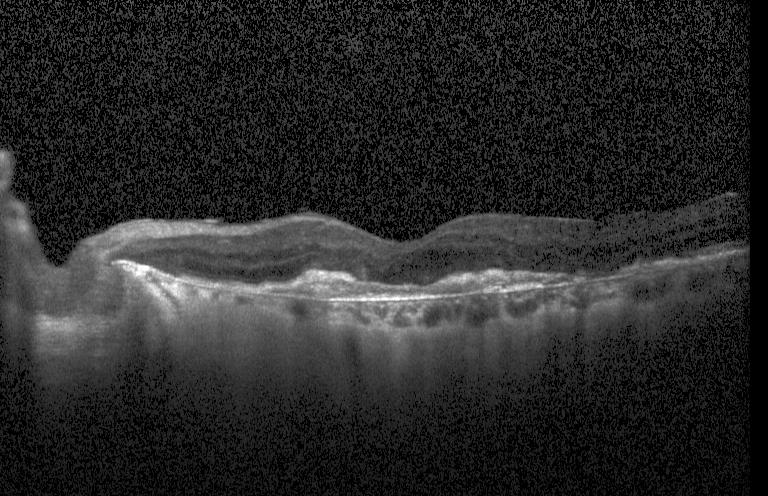 OCT finding: a choroidal neovascular membrane.